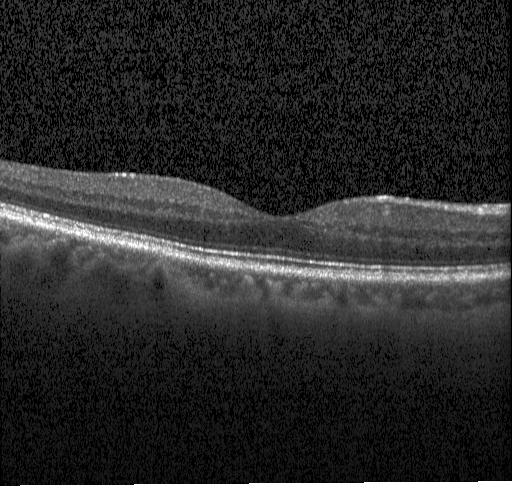
No CNV, DME, or drusen.